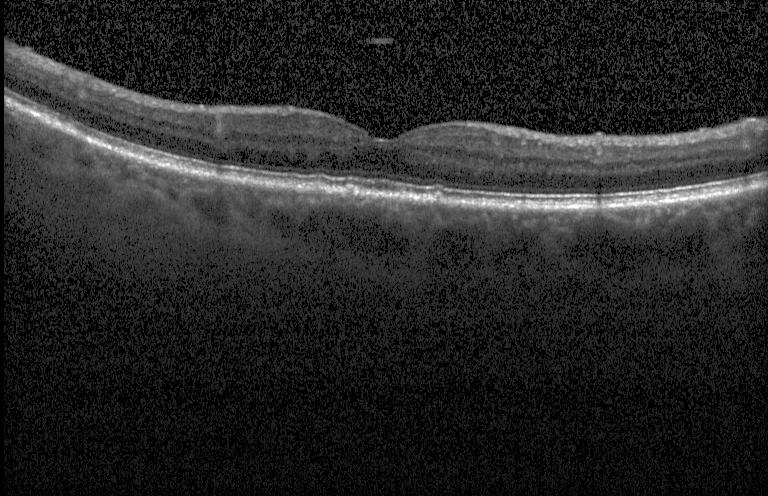 OCT line scan — Finding: multiple drusen.